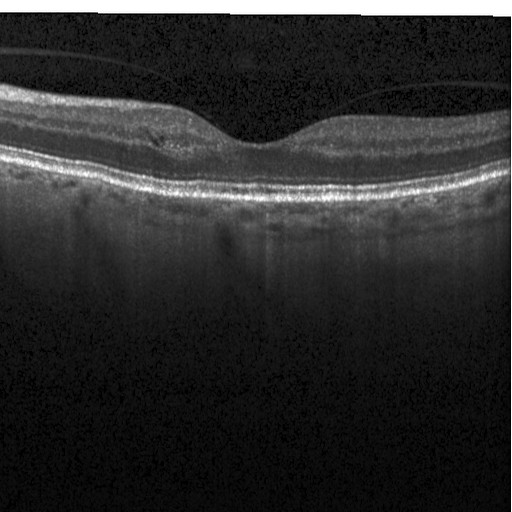
Macular OCT demonstrating diabetic macular edema.